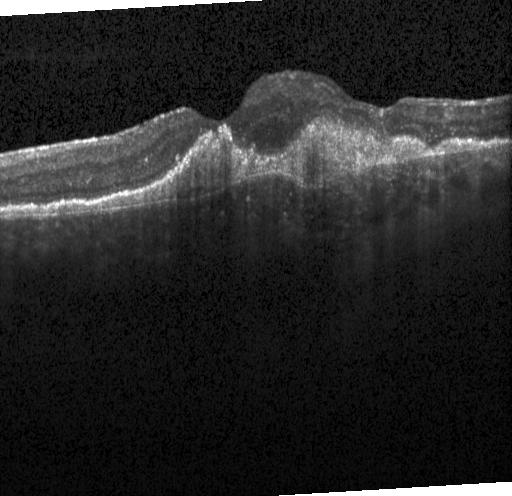 Heidelberg Spectralis · retinal OCT cross-section · macular scan.
Assessment: choroidal neovascularization.